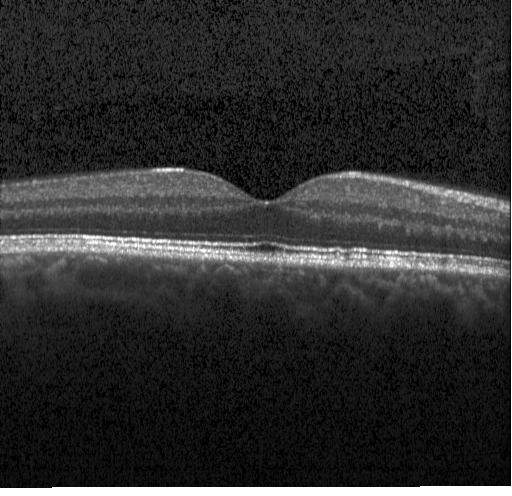 Spectral-domain optical coherence tomography · optical coherence tomography B-scan · acquired on a Heidelberg Spectralis. Assessment: no choroidal neovascularization, no diabetic macular edema, and no drusen.